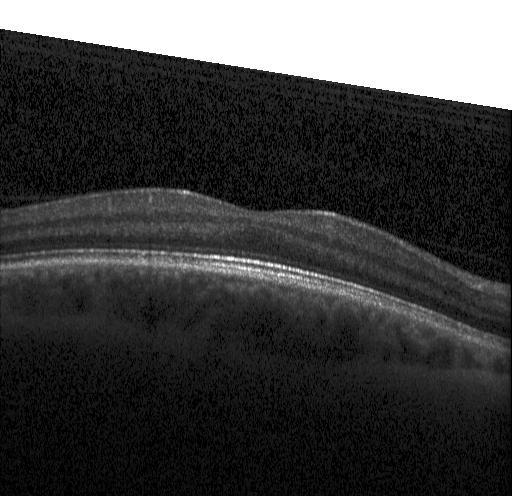 Optical coherence tomography scan.
OCT finding: no CNV, DME, or drusen.